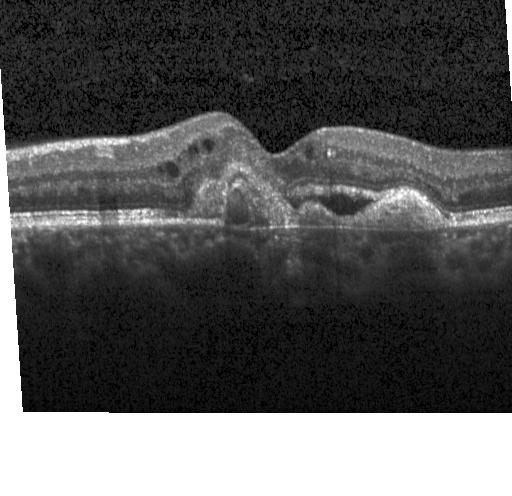 Retinal OCT B-scan · SD-OCT.
Impression: a choroidal neovascular membrane.